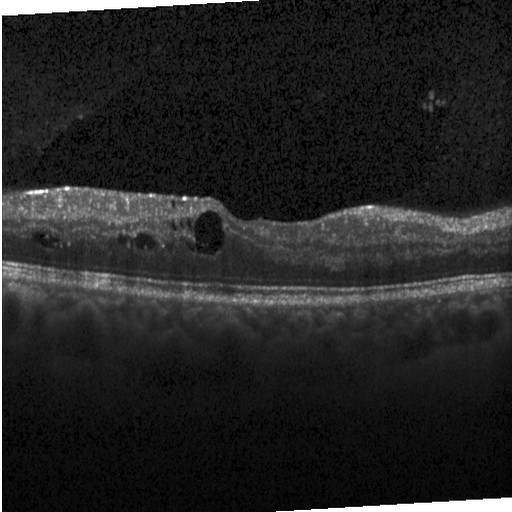

OCT B-scan — Impression: diabetic macular edema.